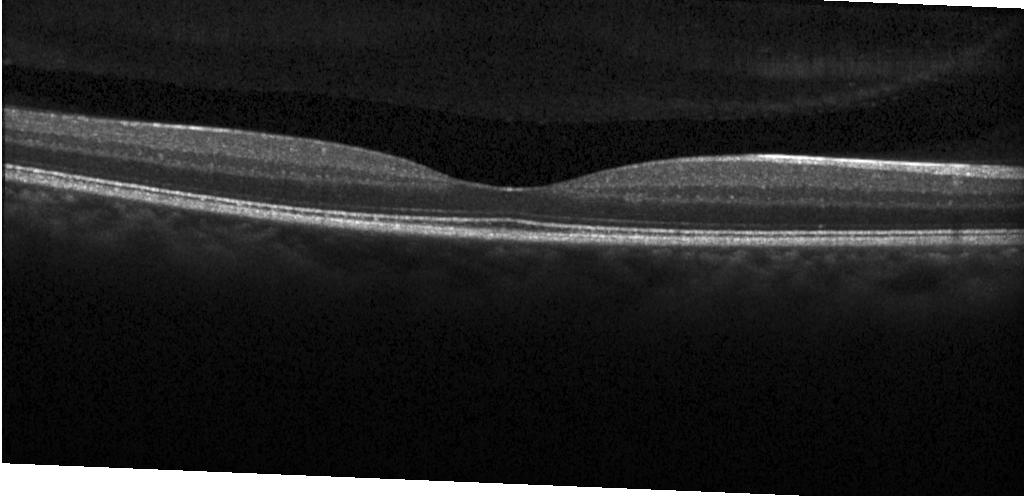

Through the macula; retinal OCT cross-section. This B-scan demonstrates no CNV, no DME, and no drusen.